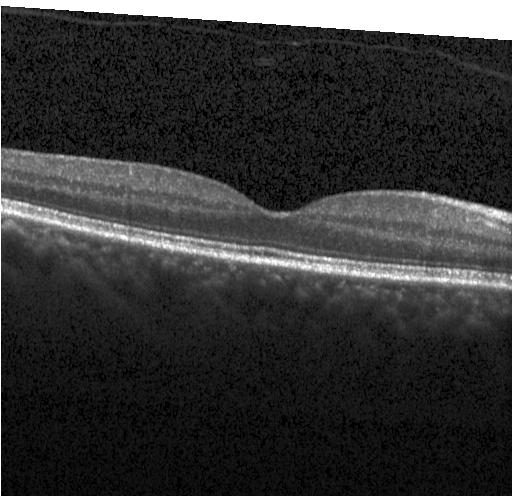 Optical coherence tomography B-scan. SD-OCT. This B-scan demonstrates no choroidal neovascularization, diabetic macular edema, or drusen.